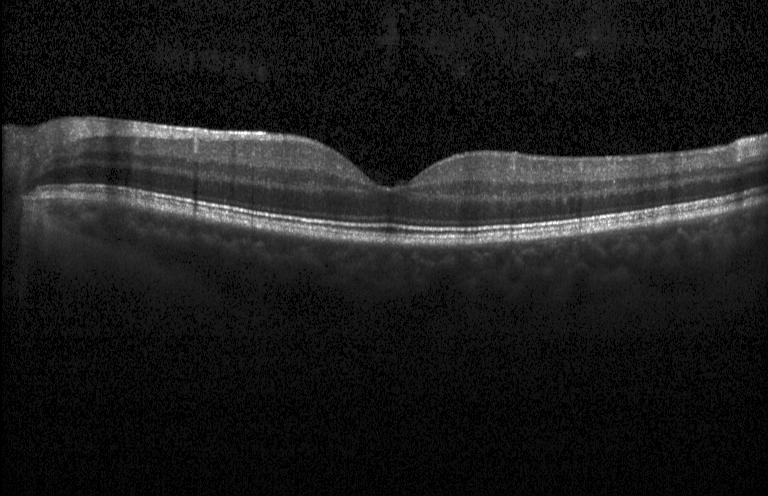

Fovea-centered · spectral-domain optical coherence tomography · Heidelberg Spectralis · retinal OCT B-scan.
Finding: no choroidal neovascularization, diabetic macular edema, or drusen.